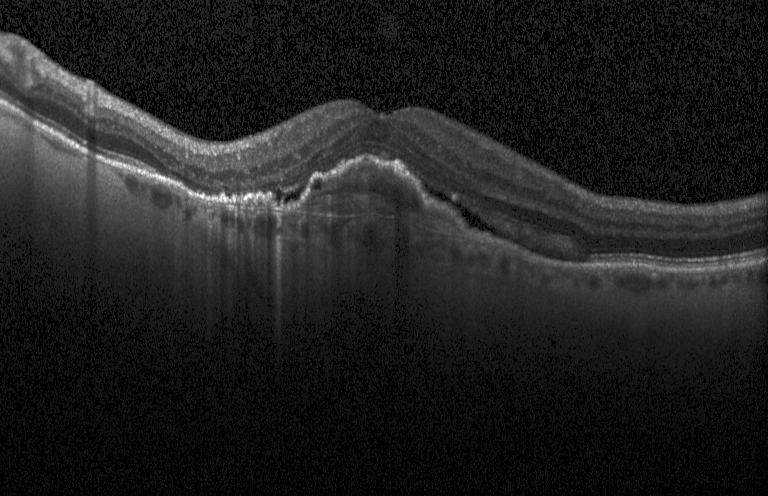 OCT line scan; through the macula; Heidelberg Spectralis; SD-OCT.
Diagnosis: CNV.